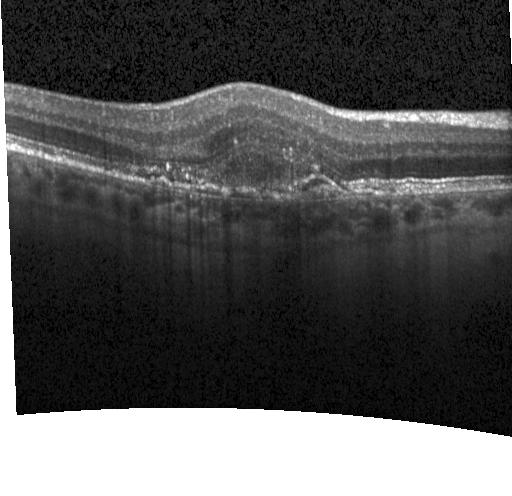

Through the macula; optical coherence tomography B-scan
Diagnosis: choroidal neovascularization.